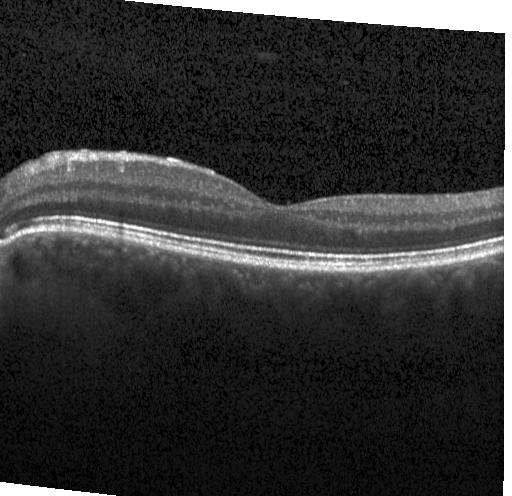

Optical coherence tomography scan.
Dx: no choroidal neovascularization, diabetic macular edema, or drusen.